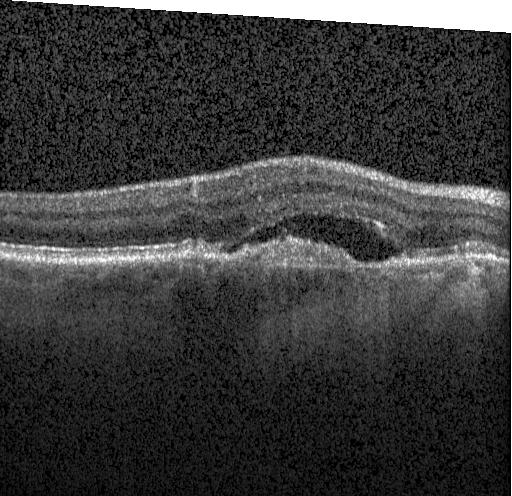 Retinal OCT cross-section.
Assessment: a choroidal neovascular membrane.